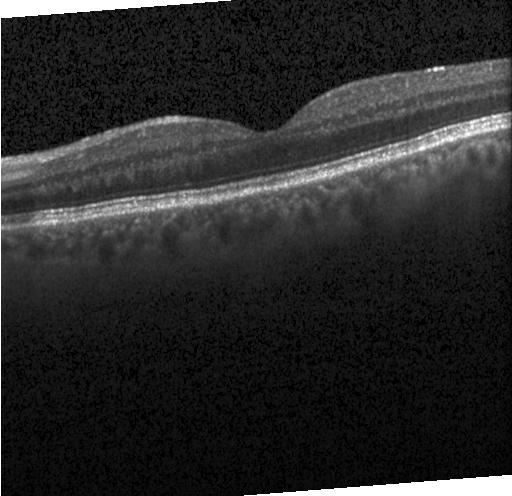 OCT line scan. Dx: no choroidal neovascularization, diabetic macular edema, or drusen.